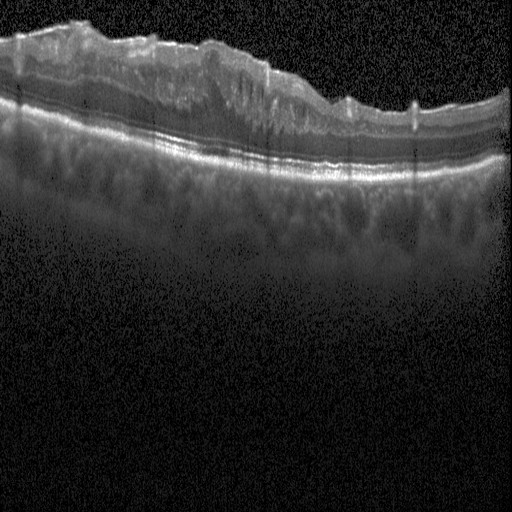
OCT line scan — Macular OCT: diabetic macular edema (DME).